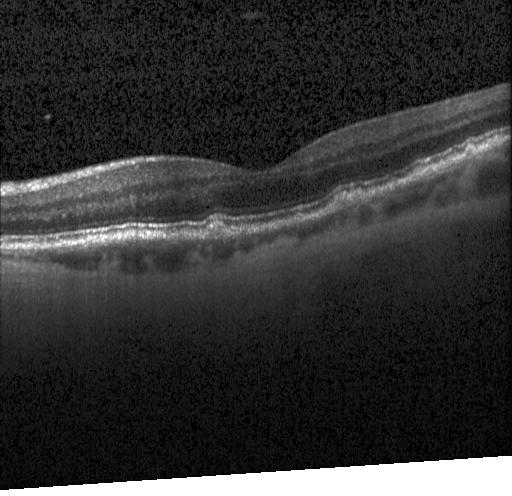
OCT B-scan; fovea-centered — Macular OCT: multiple drusen.